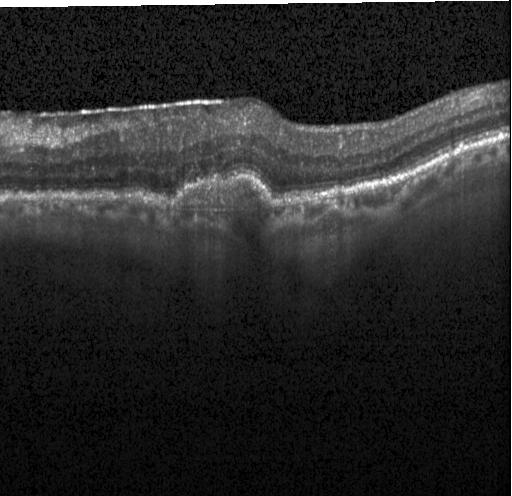
A choroidal neovascular membrane.